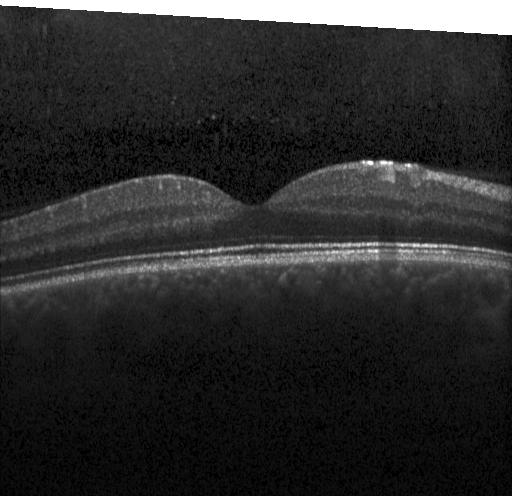 No choroidal neovascularization, no diabetic macular edema, and no drusen.